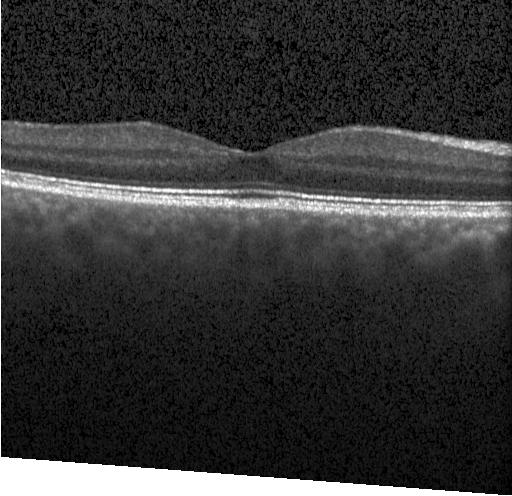
Optical coherence tomography B-scan. Dx: neither choroidal neovascularization, diabetic macular edema, nor drusen.